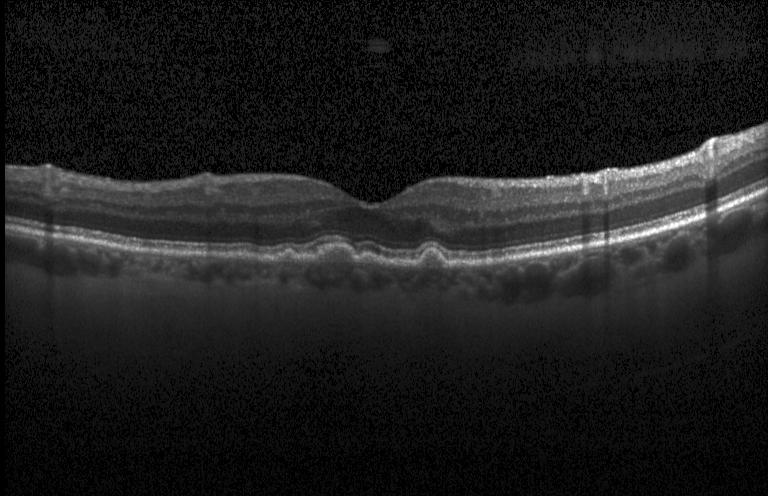

Spectral-domain OCT, retinal OCT B-scan, Heidelberg Spectralis. Macular OCT: sub-RPE drusenoid deposits.